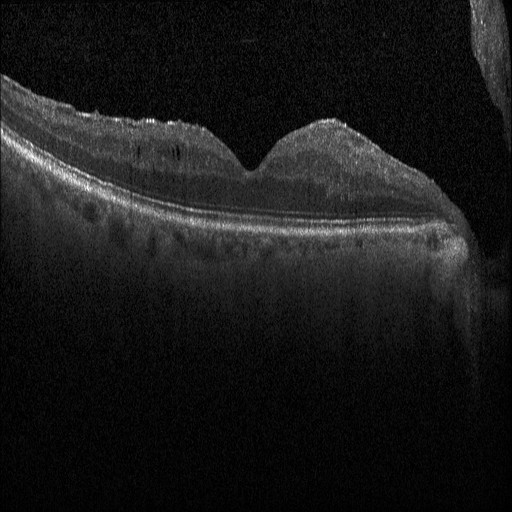 Heidelberg Spectralis; optical coherence tomography scan.
Macular OCT: diabetic macular edema (DME).